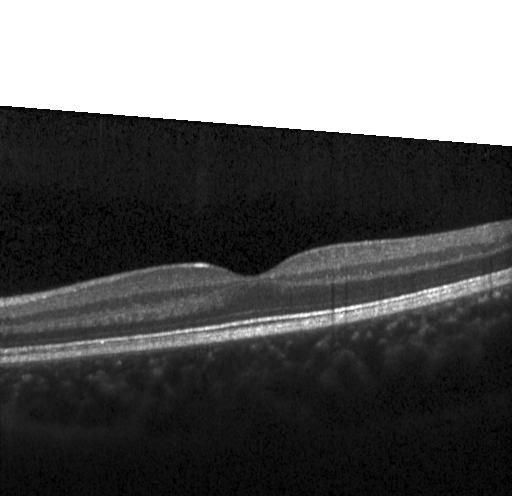
Acquired on a Heidelberg Spectralis; macular scan; spectral-domain OCT; retinal OCT cross-section
Impression: no CNV, DME, or drusen.